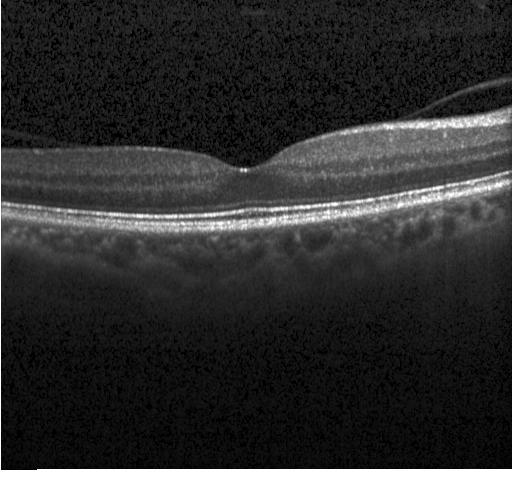

Centered on the fovea. Retinal OCT B-scan. Spectral-domain optical coherence tomography
This B-scan demonstrates neither choroidal neovascularization, diabetic macular edema, nor drusen.